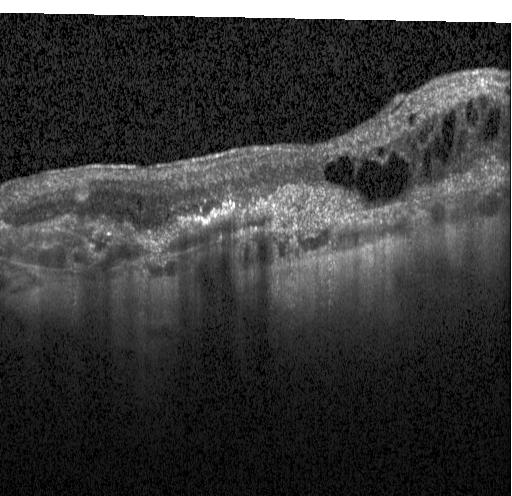 OCT finding: a choroidal neovascular membrane.